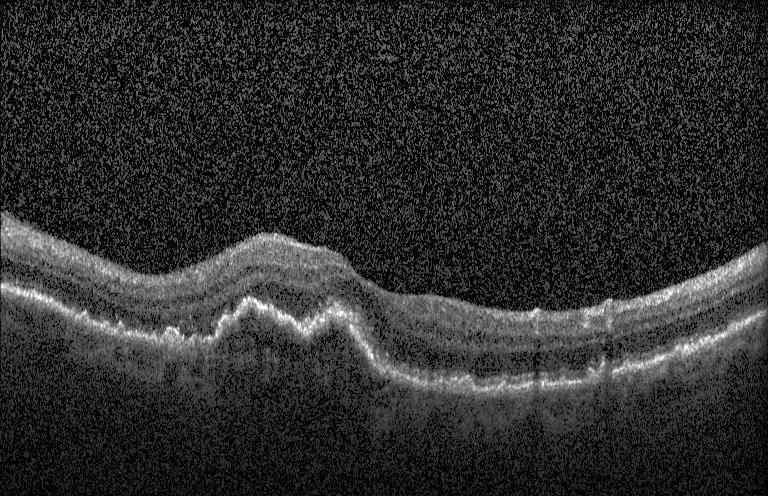
OCT B-scan — The scan shows choroidal neovascularization.